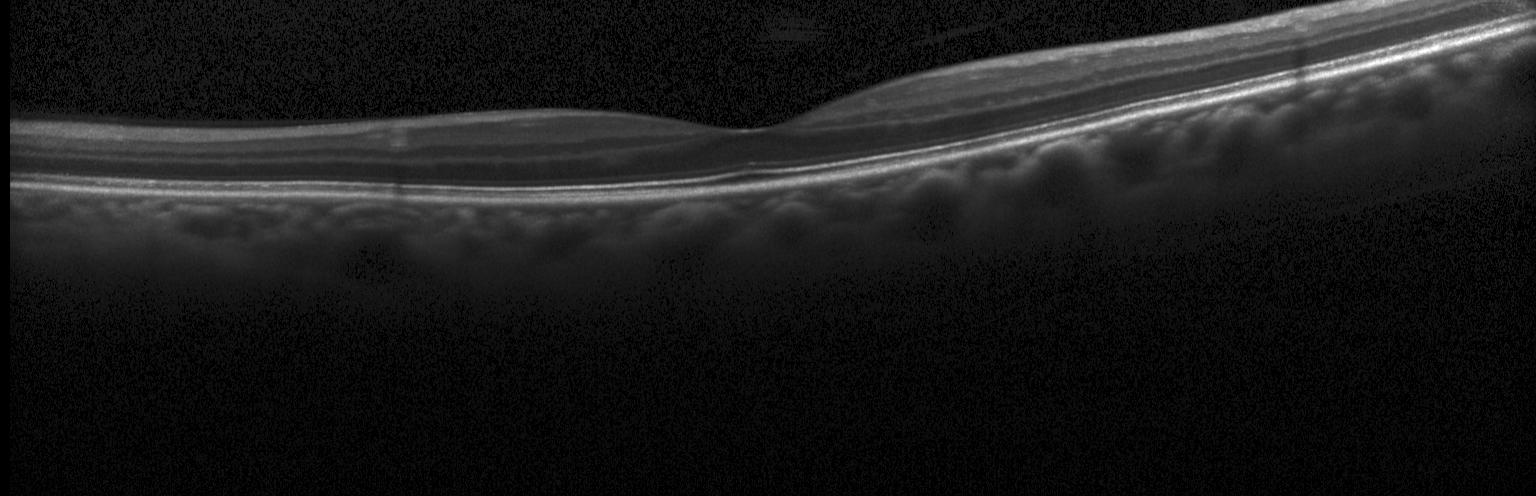 OCT B-scan · SD-OCT · Heidelberg Spectralis — Assessment: no choroidal neovascularization, no diabetic macular edema, and no drusen.